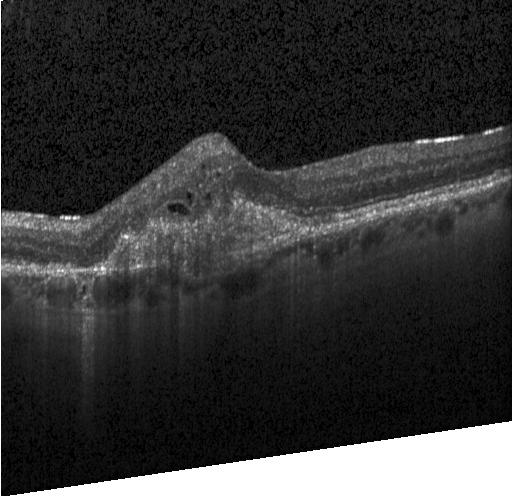

Diagnosis: choroidal neovascularization (CNV).